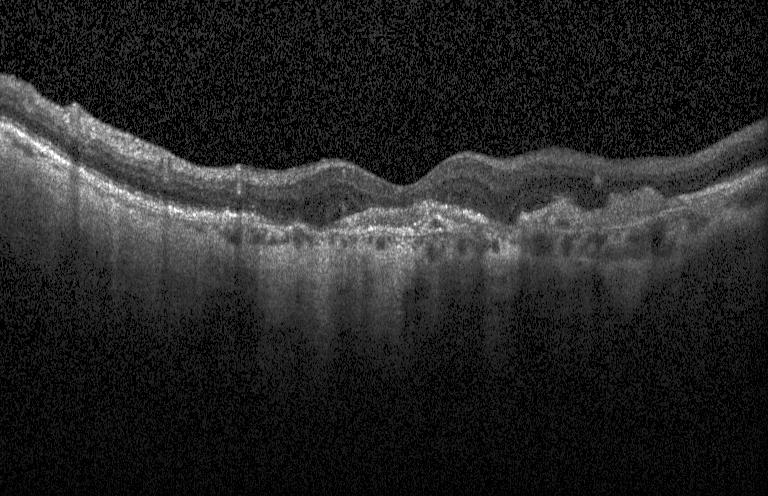 Macular scan, spectral-domain optical coherence tomography, optical coherence tomography B-scan, Heidelberg Spectralis. OCT finding: CNV.